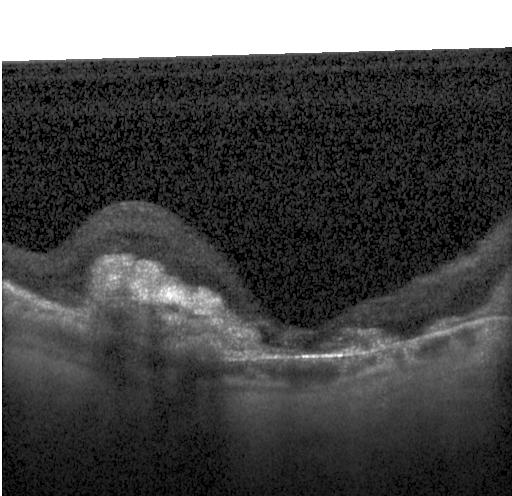 The scan shows a choroidal neovascular membrane.